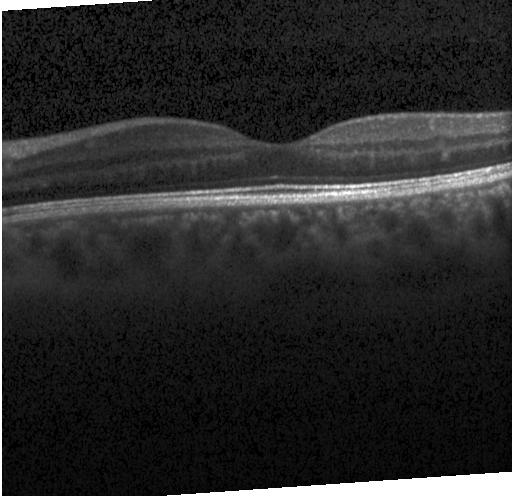

Retinal OCT B-scan. SD-OCT. Acquired on a Heidelberg Spectralis. Centered on the fovea.
This B-scan demonstrates neither CNV, DME, nor drusen.